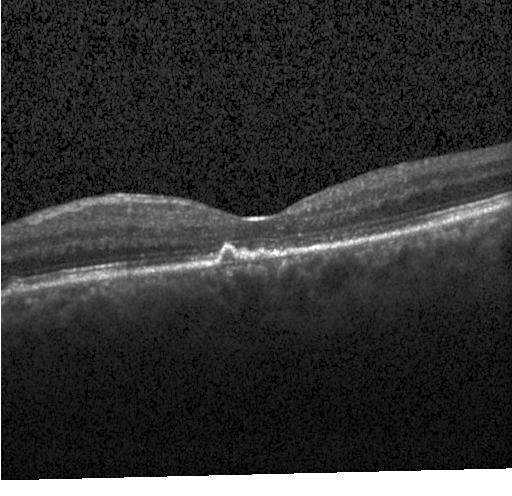 OCT B-scan. Spectral-domain OCT. Through the macula — Finding: sub-RPE drusenoid deposits.